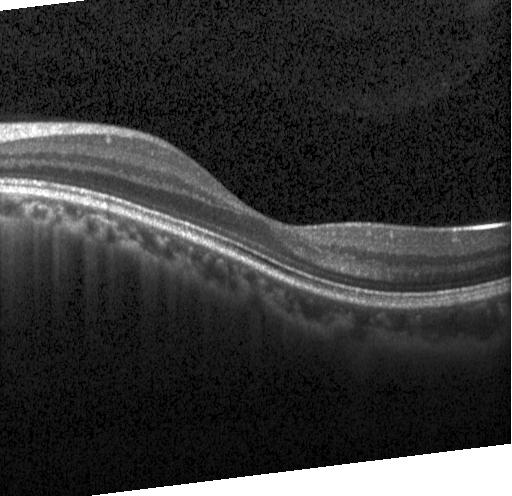 Heidelberg Spectralis OCT system, retinal OCT cross-section, spectral-domain optical coherence tomography, horizontal scan through the fovea.
This B-scan demonstrates no choroidal neovascularization, diabetic macular edema, or drusen.